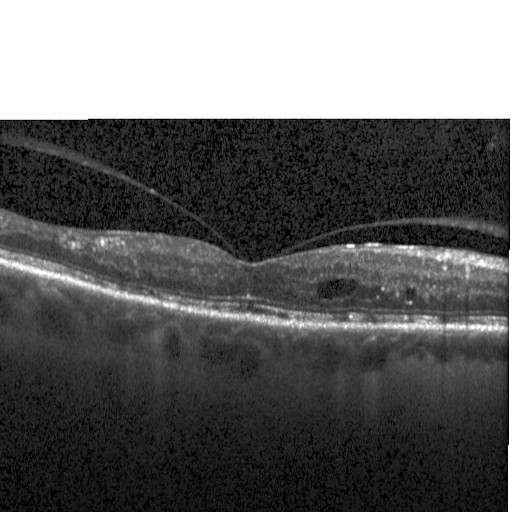
Finding: diabetic macular edema.